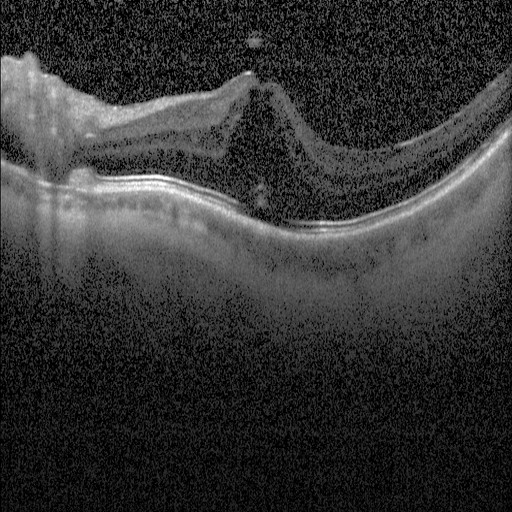 Diagnosis: diabetic macular edema.